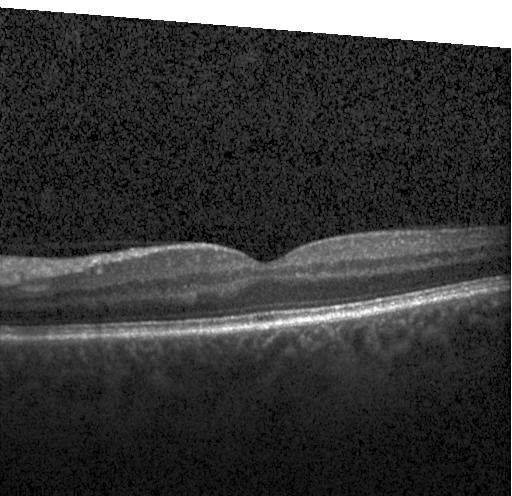

Optical coherence tomography scan. Assessment: no choroidal neovascularization, no diabetic macular edema, and no drusen.